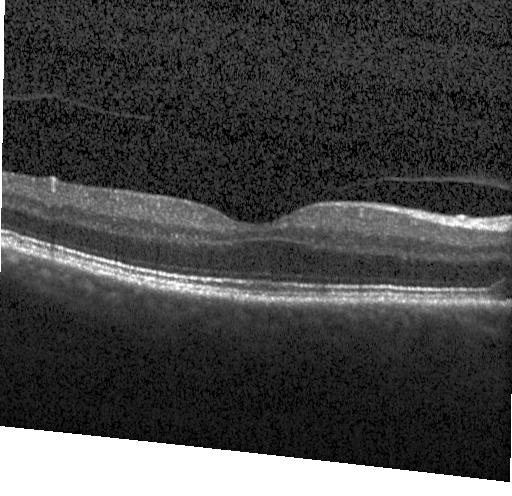
Retinal OCT cross-section — Neither choroidal neovascularization, diabetic macular edema, nor drusen.